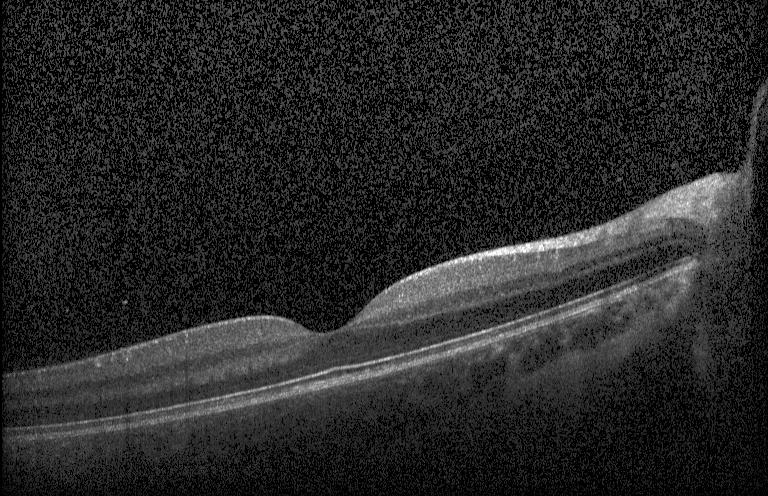 Retinal OCT B-scan. Spectral-domain OCT.
Assessment: no evidence of CNV, DME, or drusen.